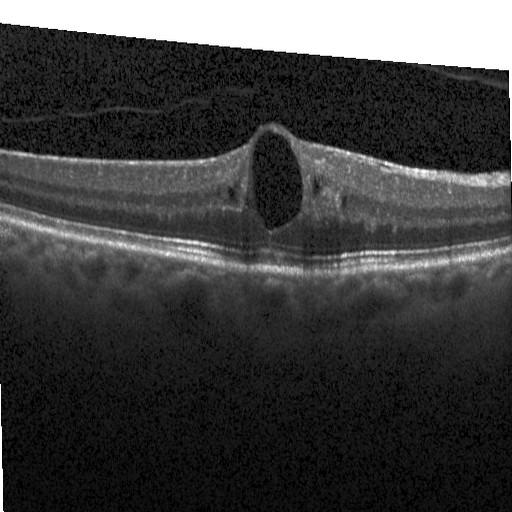

Retinal OCT B-scan, centered on the fovea, spectral-domain OCT. Diagnosis: DME.